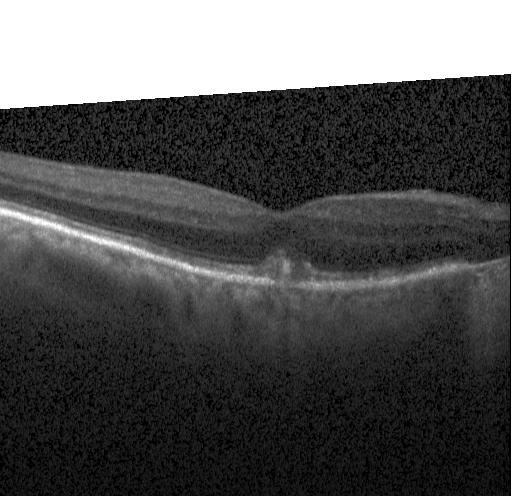 Diagnosis: a choroidal neovascular membrane.